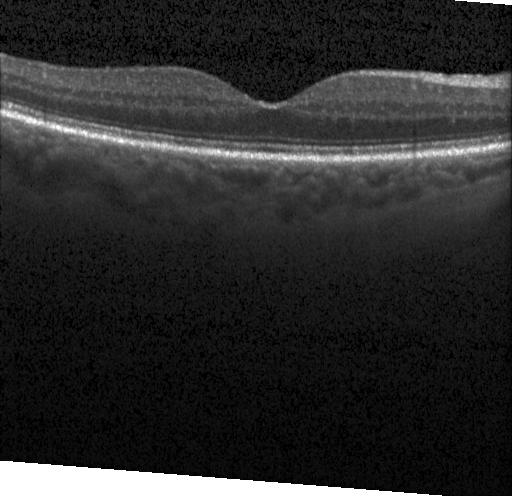 SD-OCT. OCT line scan. Through the macula. Acquired on a Heidelberg Spectralis
Diagnosis: no choroidal neovascularization, no diabetic macular edema, and no drusen.